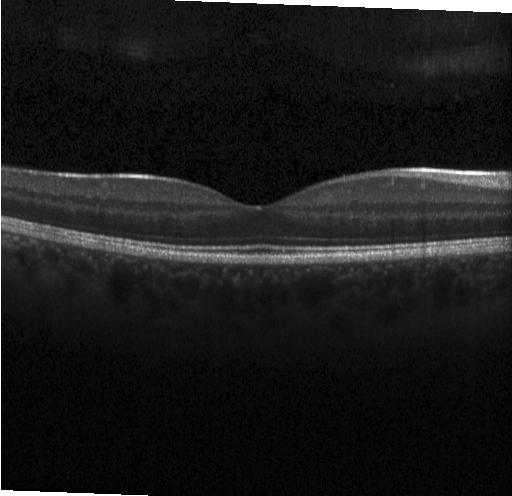 Assessment: no evidence of choroidal neovascularization, diabetic macular edema, or drusen.